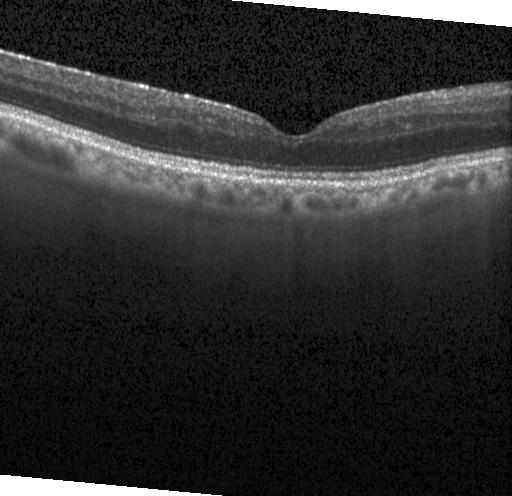
Spectral-domain optical coherence tomography; optical coherence tomography B-scan; Heidelberg Spectralis OCT system; fovea-centered.
OCT finding: no choroidal neovascularization, diabetic macular edema, or drusen.